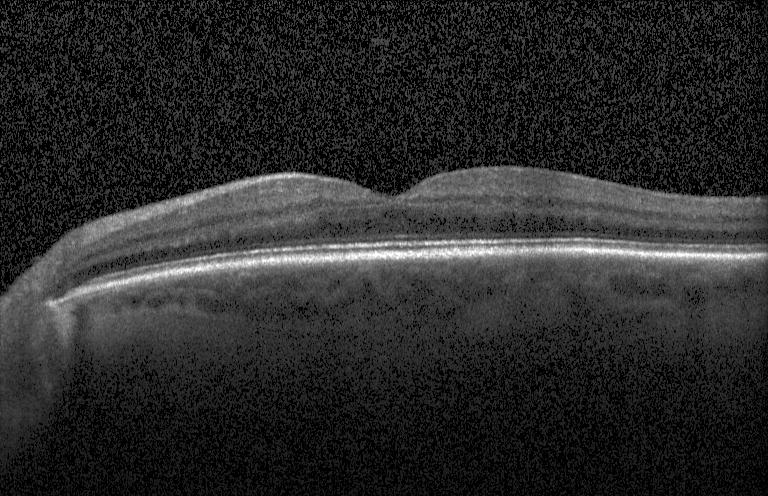

SD-OCT. Optical coherence tomography B-scan.
Impression: no CNV, DME, or drusen.